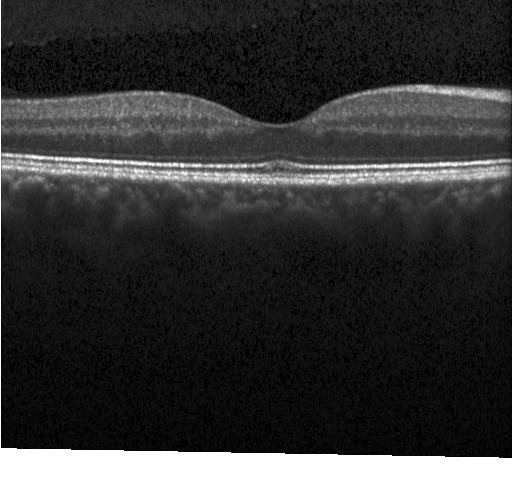
Optical coherence tomography scan; spectral-domain optical coherence tomography; fovea-centered; acquired on a Heidelberg Spectralis. Assessment: no CNV, no DME, and no drusen.